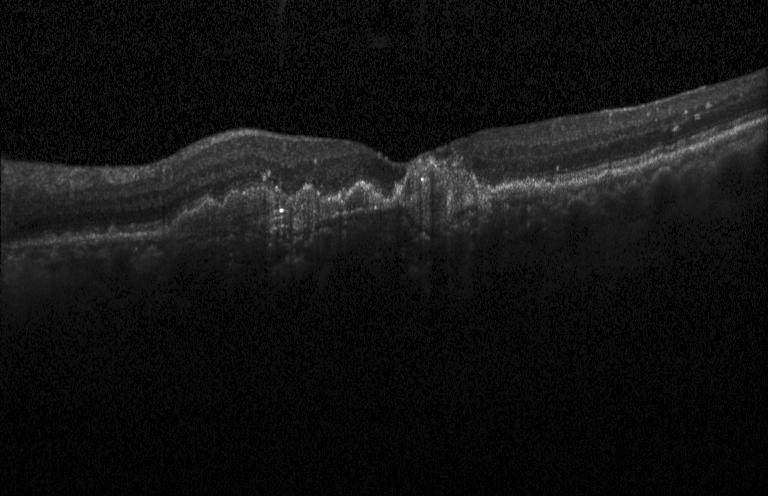 Macular OCT demonstrating choroidal neovascularization.